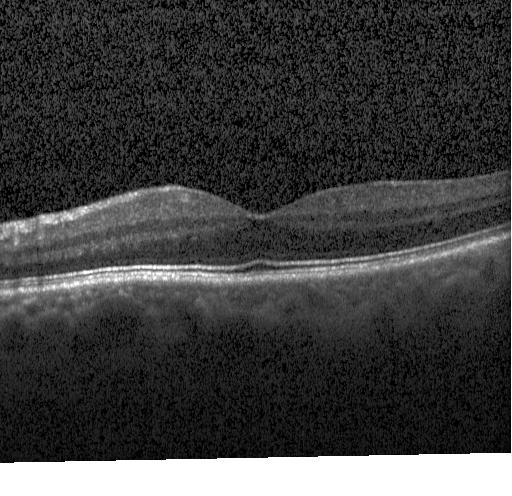

Finding: no evidence of choroidal neovascularization, diabetic macular edema, or drusen.